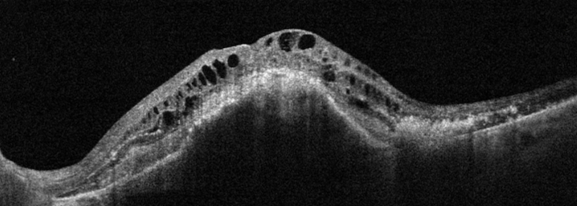
OCT B-scan
OCT finding: AMD.